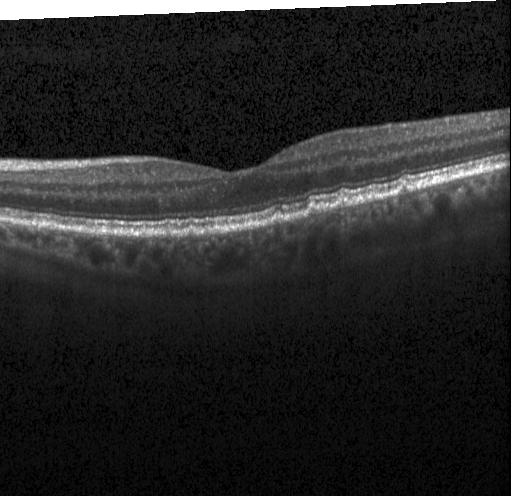

OCT B-scan
Dx: sub-RPE drusenoid deposits.